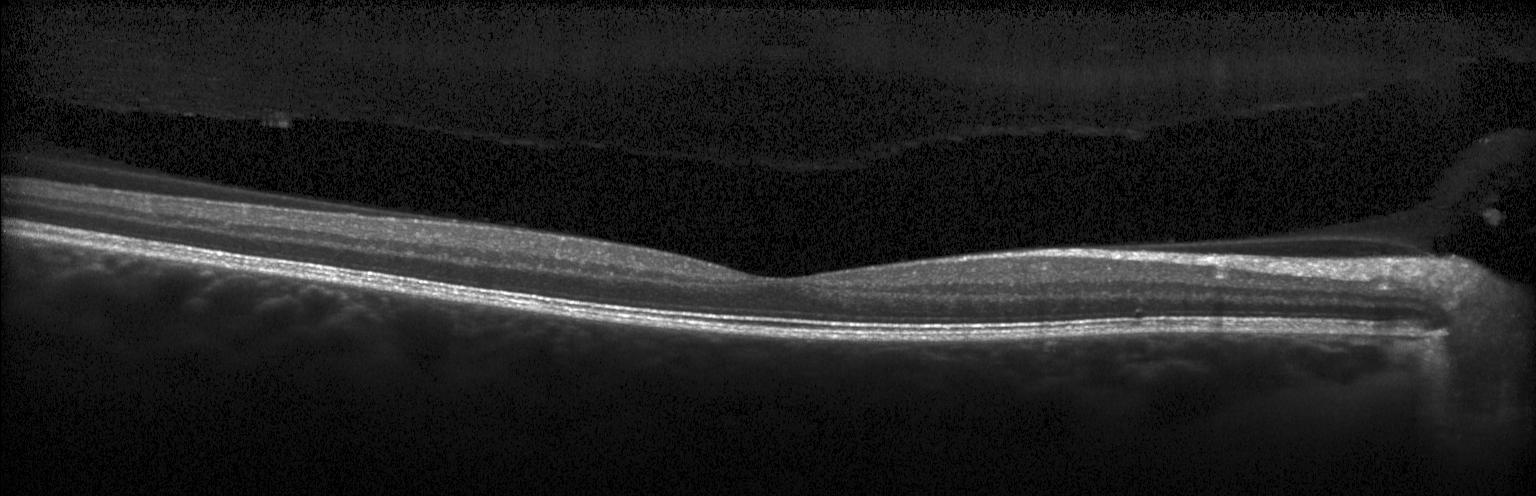 Retinal OCT B-scan — Diagnosis: no evidence of CNV, DME, or drusen.